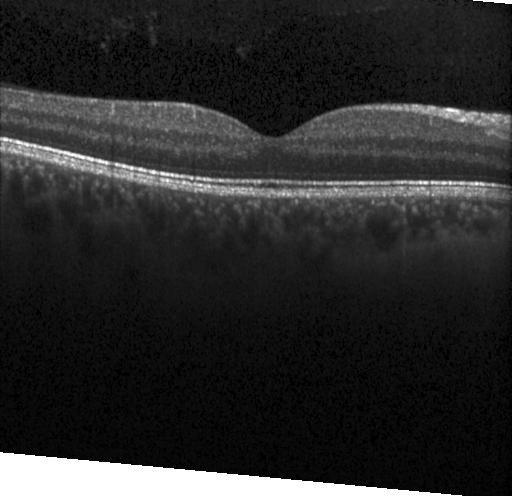

Optical coherence tomography scan — Finding: no choroidal neovascularization, no diabetic macular edema, and no drusen.